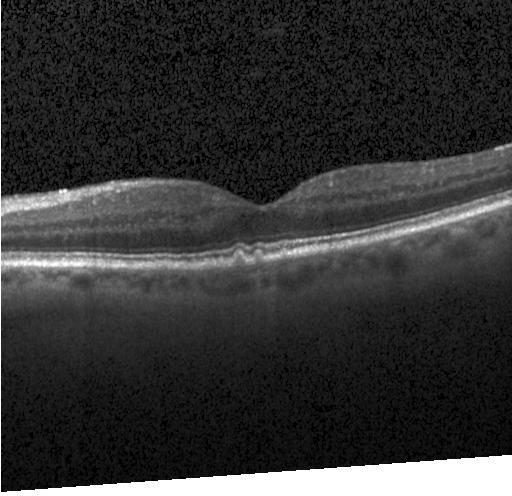 OCT line scan. Heidelberg Spectralis OCT system. SD-OCT.
The scan shows multiple drusen.